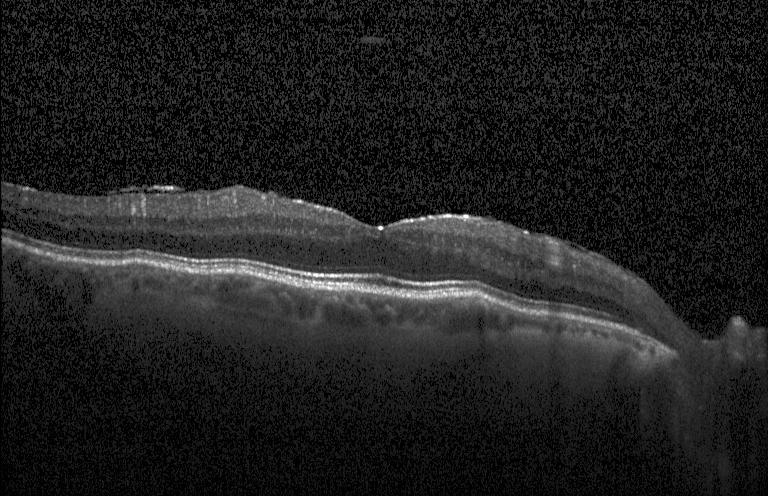
OCT line scan · centered on the fovea.
This B-scan demonstrates no CNV, no DME, and no drusen.